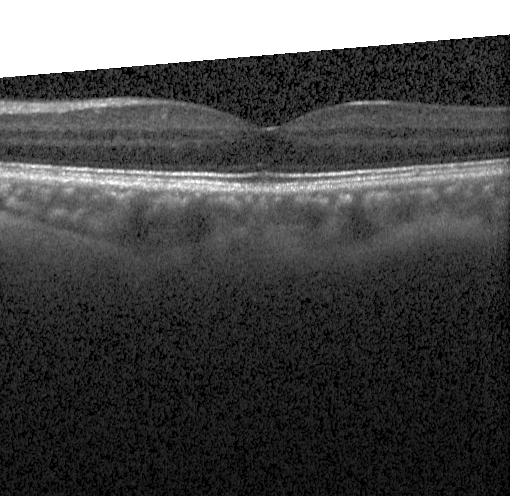
Retinal OCT B-scan
OCT finding: no evidence of choroidal neovascularization, diabetic macular edema, or drusen.